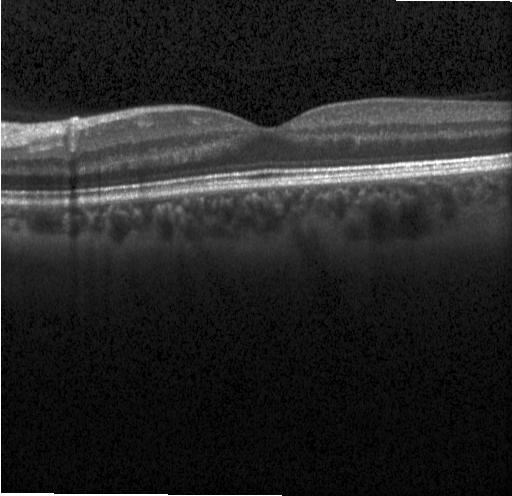
Optical coherence tomography B-scan. Spectral-domain OCT. Acquired on a Heidelberg Spectralis. Macular scan
This B-scan demonstrates no choroidal neovascularization, no diabetic macular edema, and no drusen.